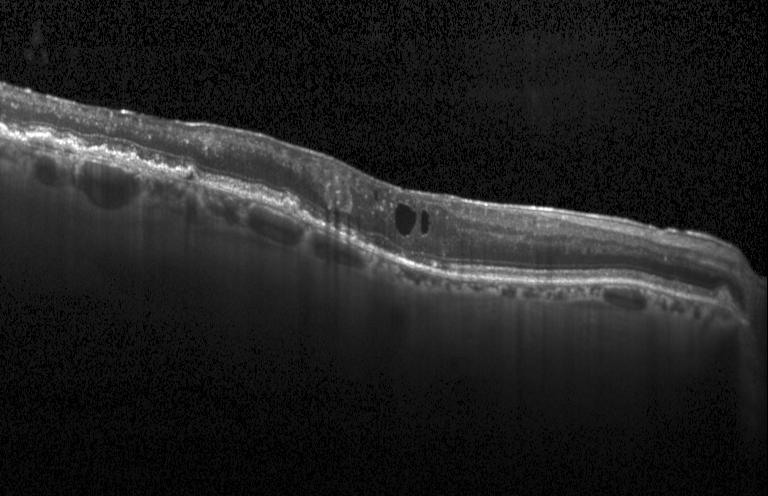 Heidelberg Spectralis. Optical coherence tomography scan
This B-scan demonstrates a choroidal neovascular membrane.